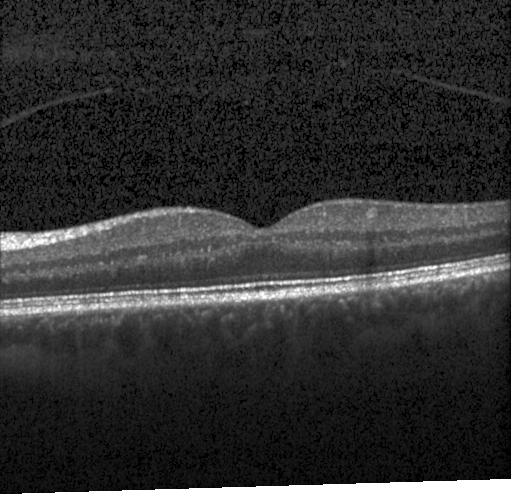

Optical coherence tomography B-scan — Assessment: no choroidal neovascularization, no diabetic macular edema, and no drusen.